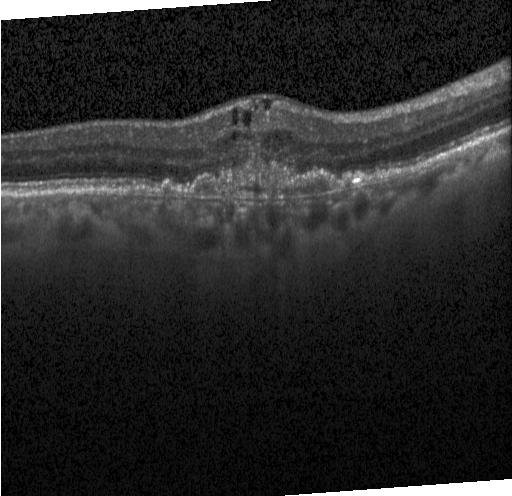 Optical coherence tomography scan. Through the macula. Acquired on a Heidelberg Spectralis.
Impression: choroidal neovascularization.